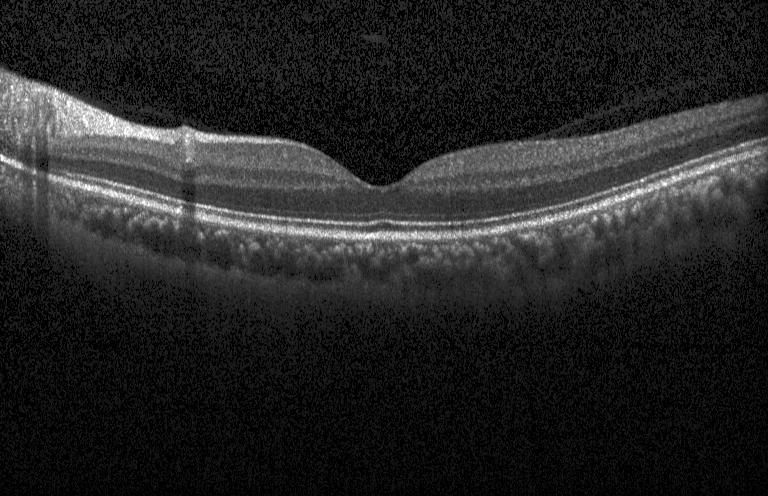 Instrument: Heidelberg Spectralis. Retinal OCT B-scan. Macular scan — Macular OCT: no choroidal neovascularization, no diabetic macular edema, and no drusen.